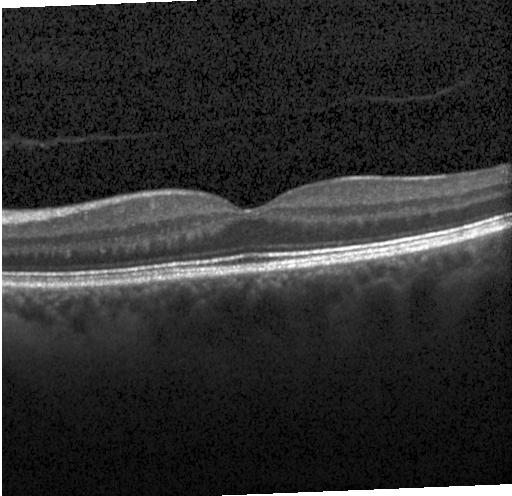
Macular scan, OCT line scan, instrument: Heidelberg Spectralis, SD-OCT.
Macular OCT: neither CNV, DME, nor drusen.